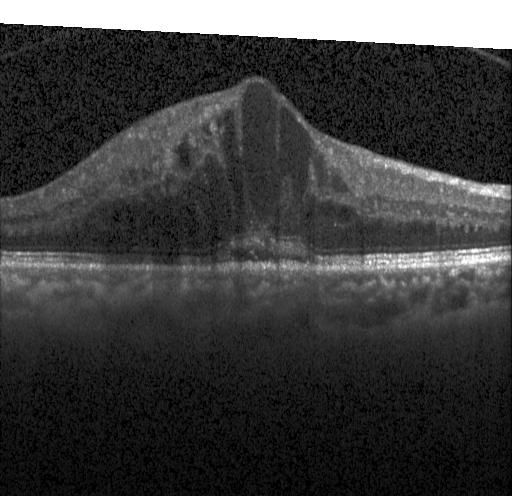 Horizontal scan through the fovea · instrument: Heidelberg Spectralis · OCT B-scan · SD-OCT. Assessment: diabetic macular edema.